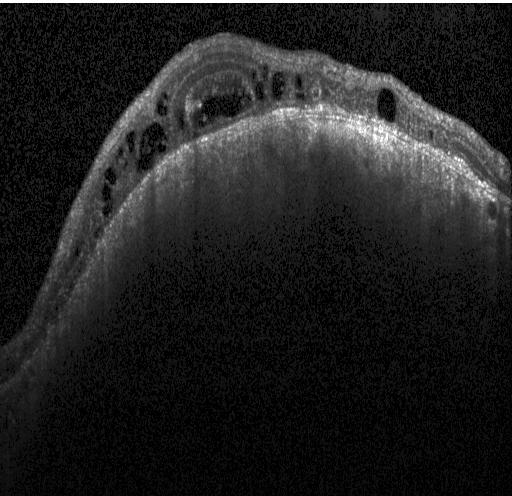 Optical coherence tomography scan. Through the macula. Impression: diabetic macular edema.